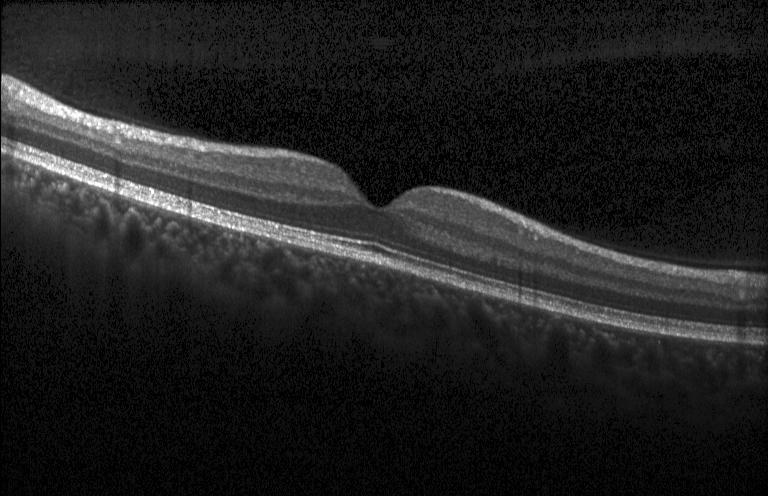
Impression: no evidence of choroidal neovascularization, diabetic macular edema, or drusen.